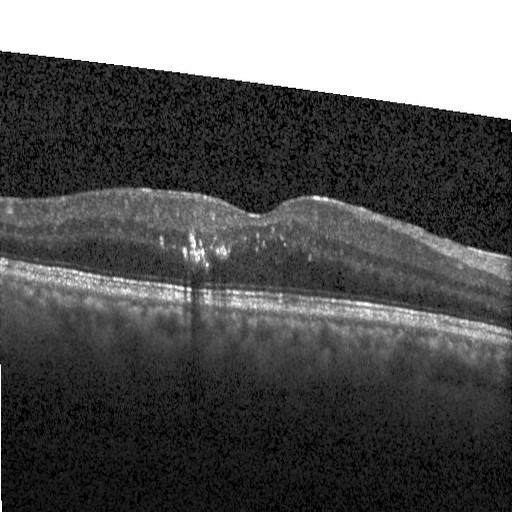
Diagnosis: diabetic macular edema.